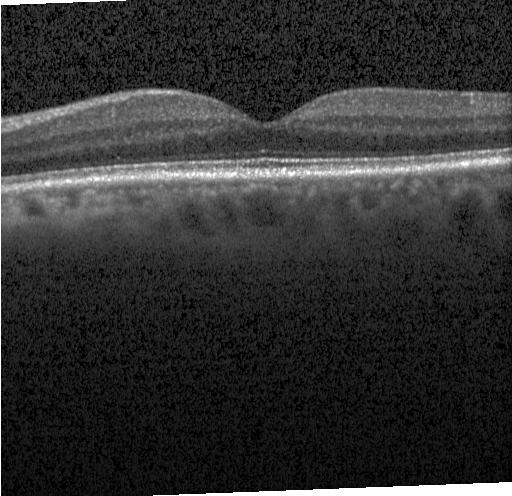

Optical coherence tomography scan · spectral-domain OCT · horizontal scan through the fovea · acquired on a Heidelberg Spectralis — Assessment: no choroidal neovascularization, diabetic macular edema, or drusen.